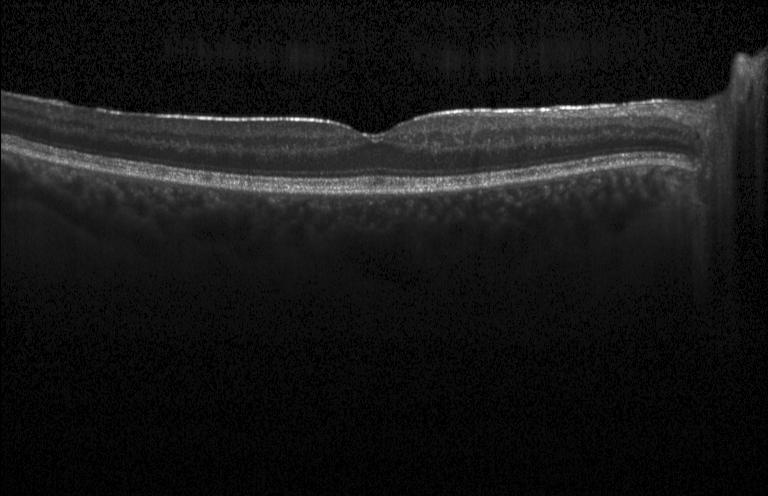
Spectral-domain optical coherence tomography. Instrument: Heidelberg Spectralis. Optical coherence tomography scan. Assessment: neither choroidal neovascularization, diabetic macular edema, nor drusen.